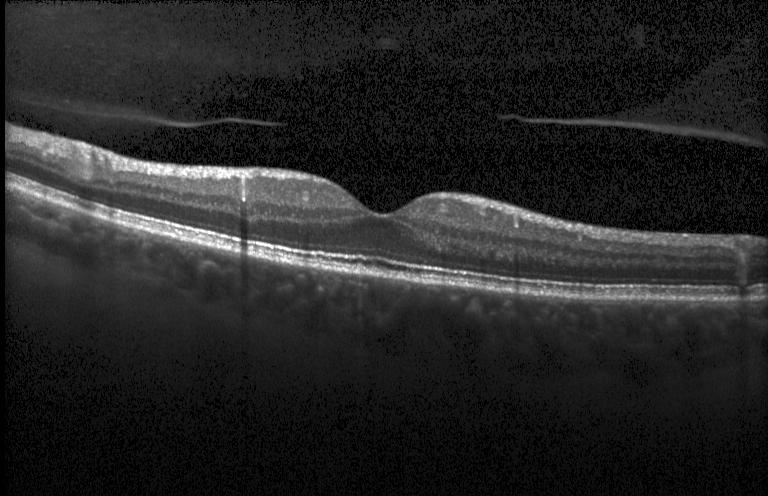 Macular OCT: no choroidal neovascularization, diabetic macular edema, or drusen.